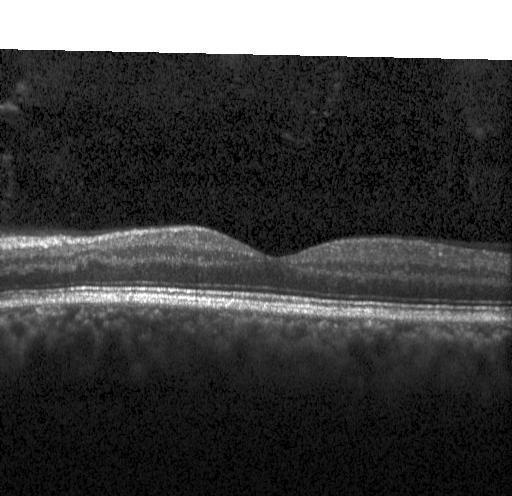
Optical coherence tomography scan · fovea-centered. Neither CNV, DME, nor drusen.